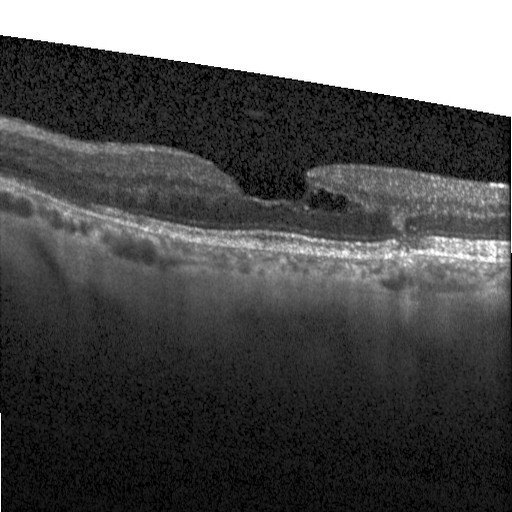 Optical coherence tomography B-scan; Heidelberg Spectralis; spectral-domain OCT.
This B-scan demonstrates diabetic macular edema (DME).